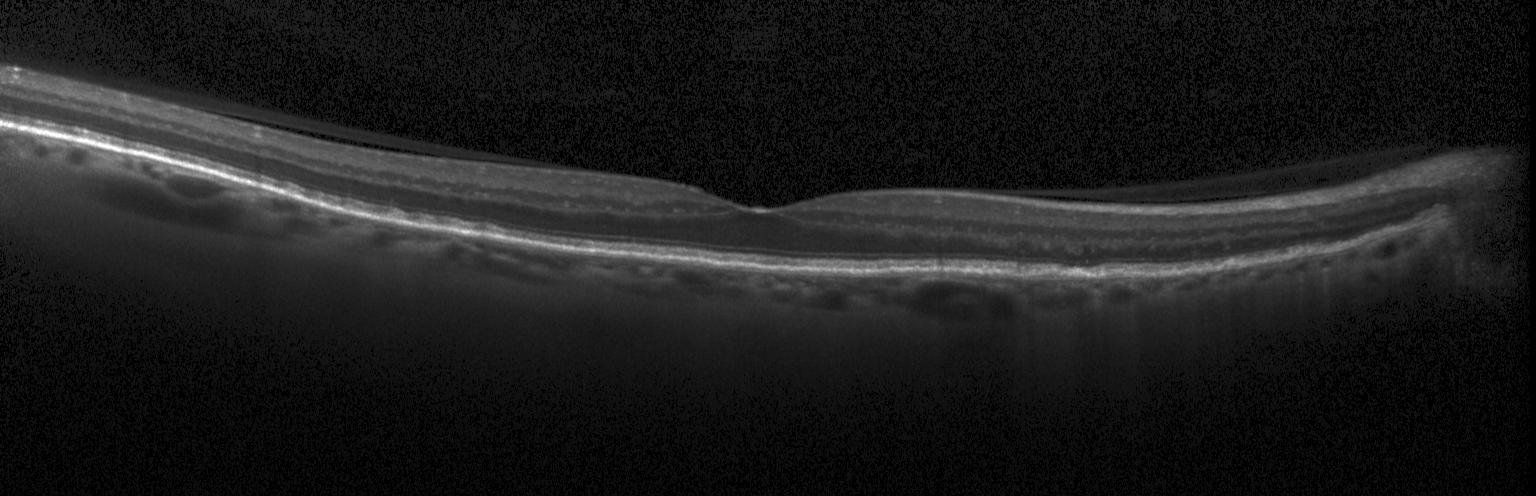
Assessment: neither choroidal neovascularization, diabetic macular edema, nor drusen.